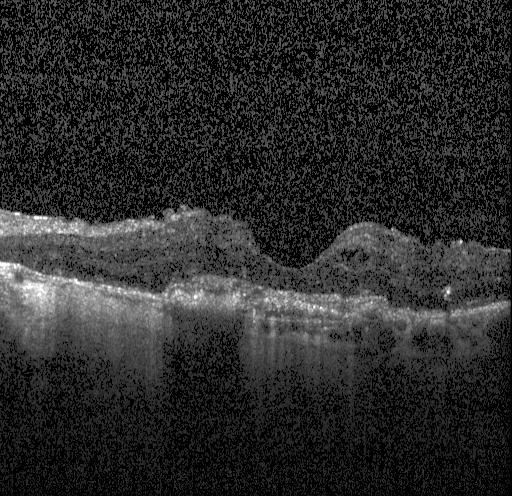
Retinal OCT cross-section showing CNV.